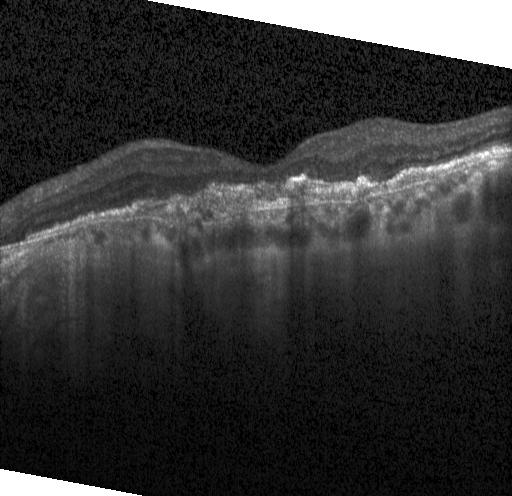
OCT B-scan — Diagnosis: choroidal neovascularization.